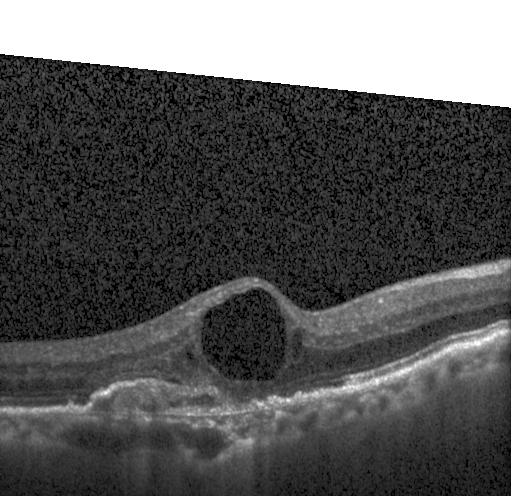
OCT B-scan. Acquired on a Heidelberg Spectralis
Finding: a choroidal neovascular membrane.